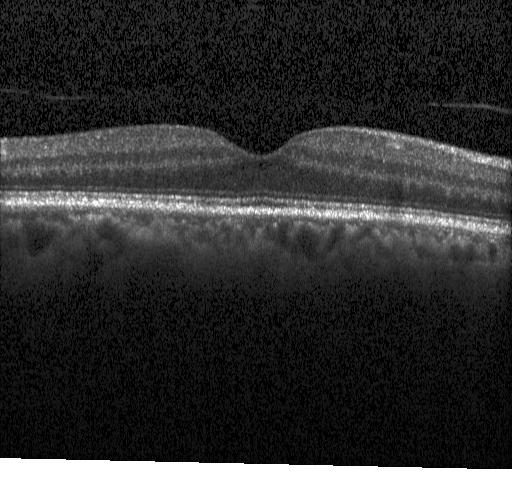

Retinal OCT cross-section
Diagnosis: no choroidal neovascularization, diabetic macular edema, or drusen.